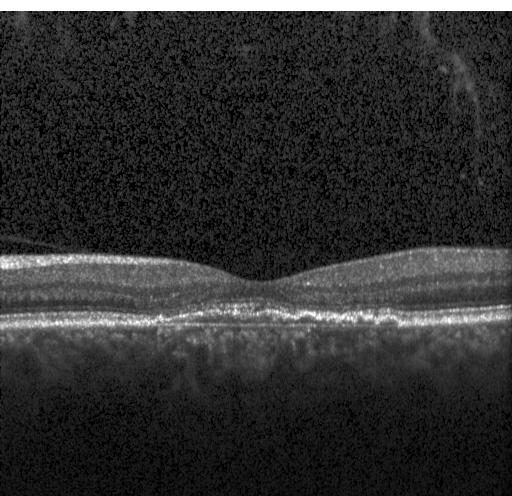
Centered on the fovea · instrument: Heidelberg Spectralis · optical coherence tomography B-scan.
Dx: CNV.